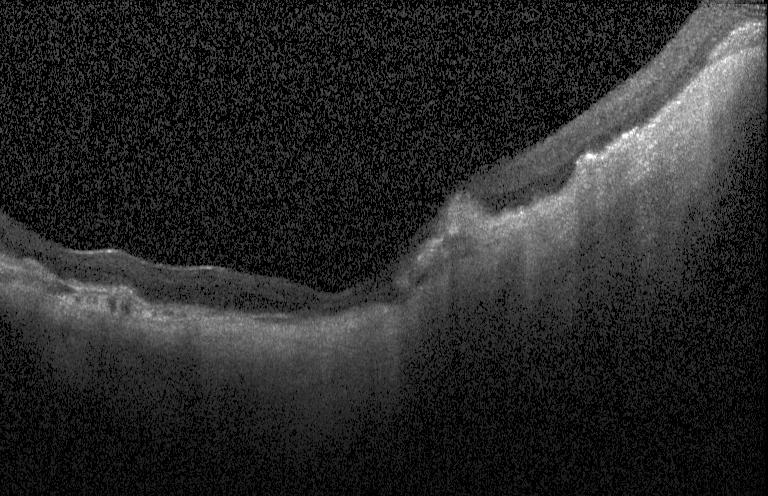
Dx: choroidal neovascularization.